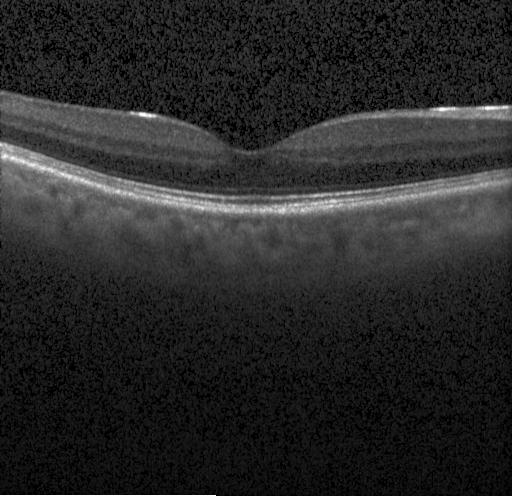
OCT scan showing neither choroidal neovascularization, diabetic macular edema, nor drusen.